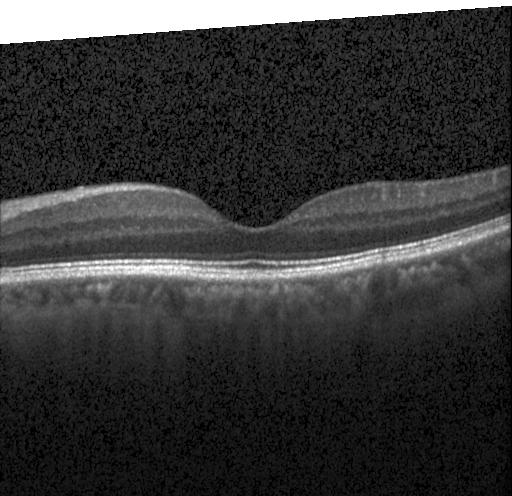
Retinal OCT cross-section showing no evidence of CNV, DME, or drusen.